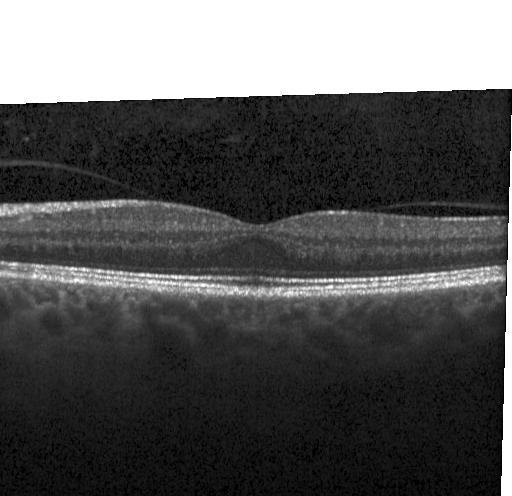

Neither CNV, DME, nor drusen.